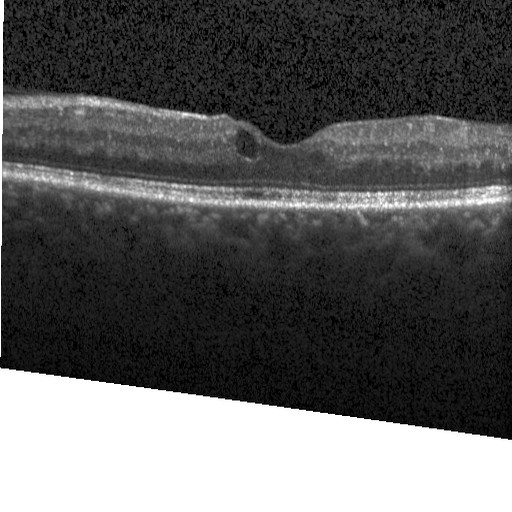

Acquired on a Heidelberg Spectralis; OCT B-scan; centered on the fovea; SD-OCT — Impression: DME.